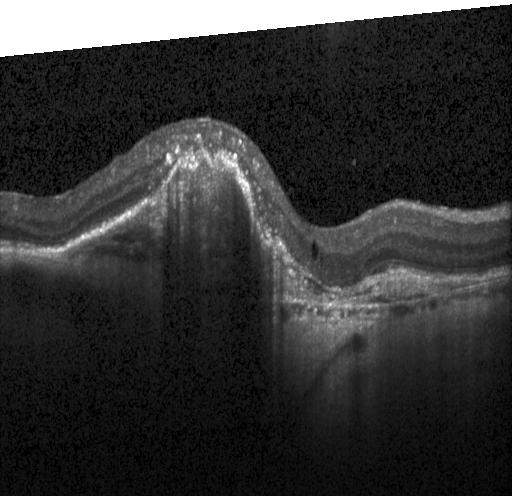
Diagnosis: choroidal neovascularization.